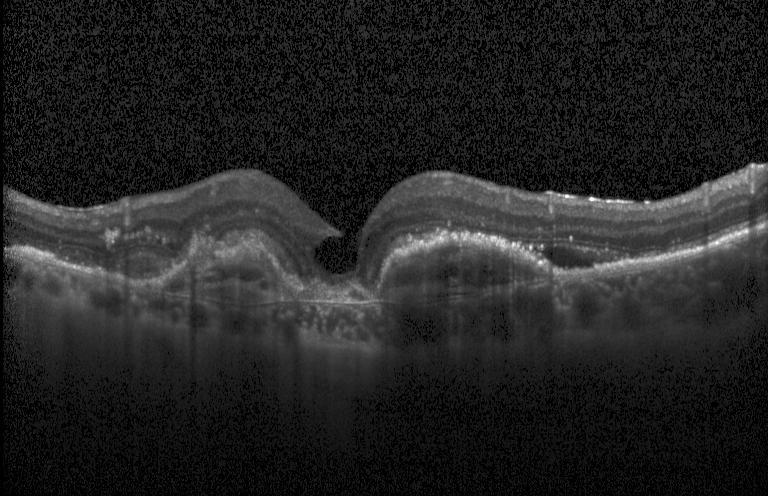 Retinal OCT B-scan. Centered on the fovea. Spectral-domain optical coherence tomography — This B-scan demonstrates CNV.